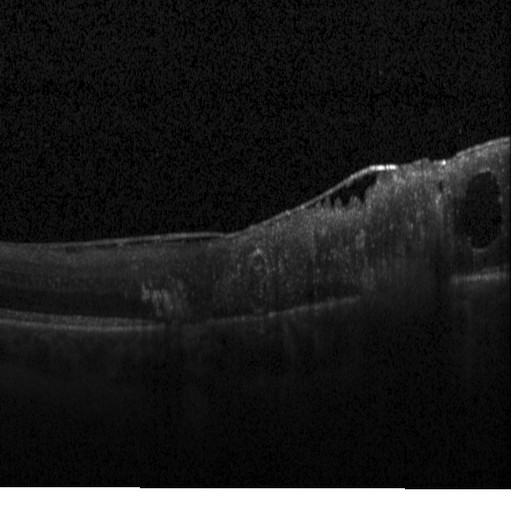

Finding: DME.